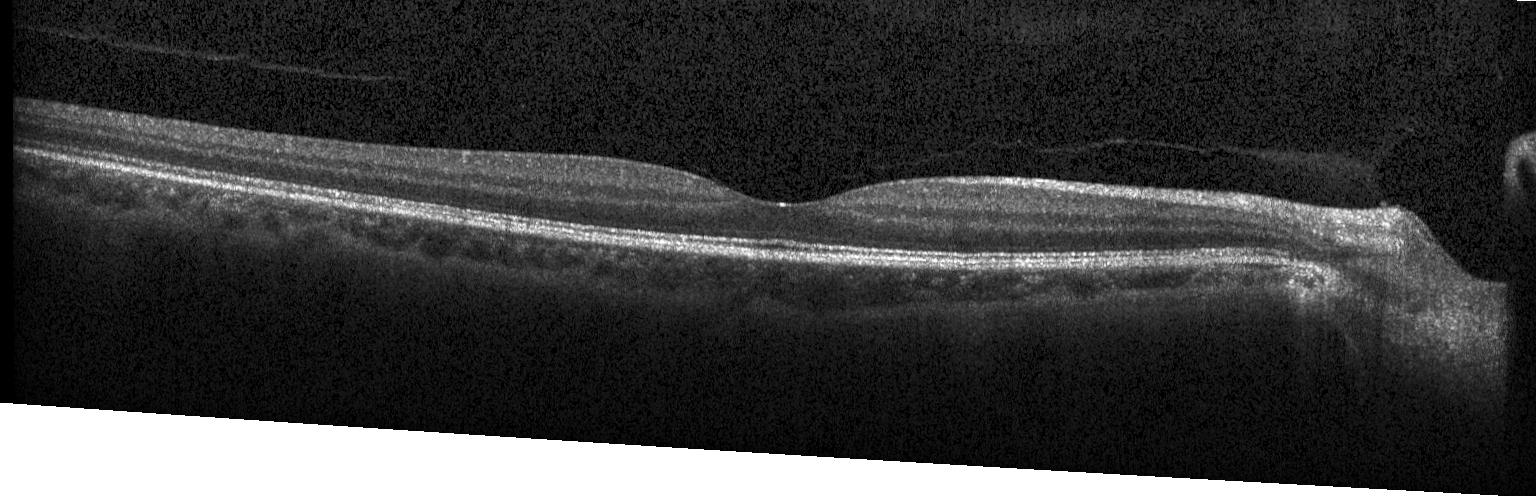
Impression: no choroidal neovascularization, diabetic macular edema, or drusen.